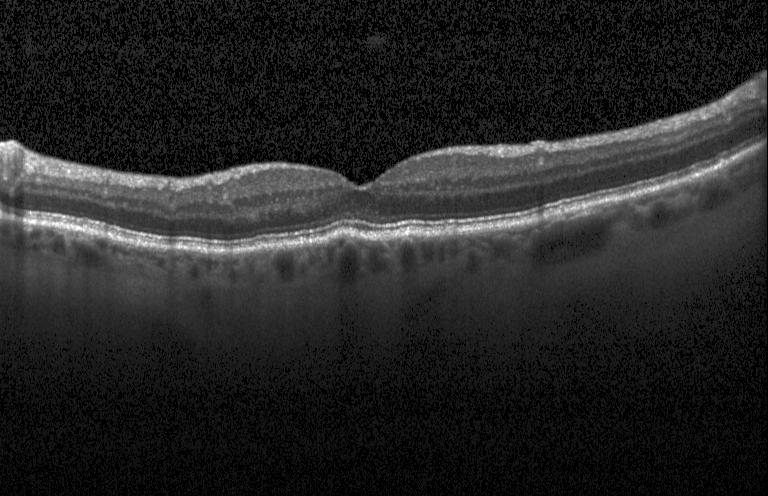

Spectral-domain OCT B-scan: no choroidal neovascularization, no diabetic macular edema, and no drusen.